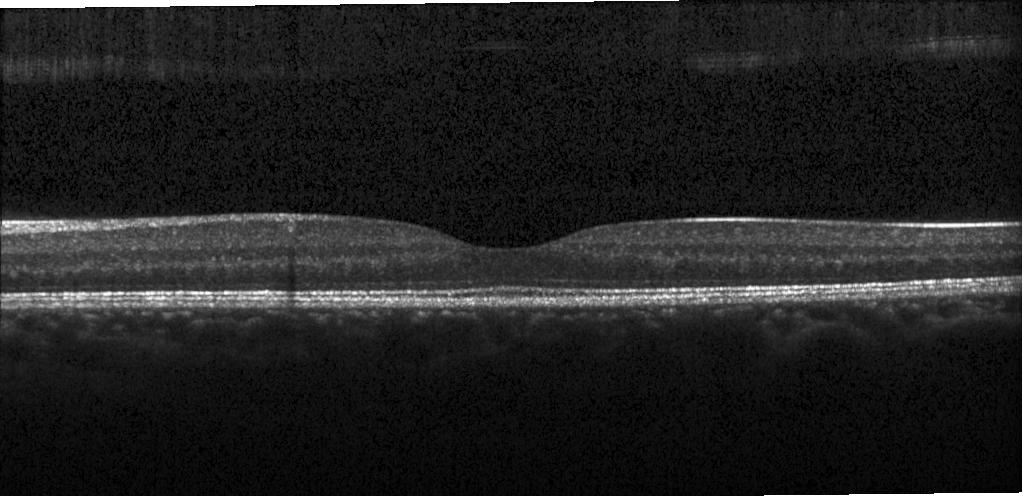

Retinal OCT cross-section
This B-scan demonstrates no evidence of choroidal neovascularization, diabetic macular edema, or drusen.